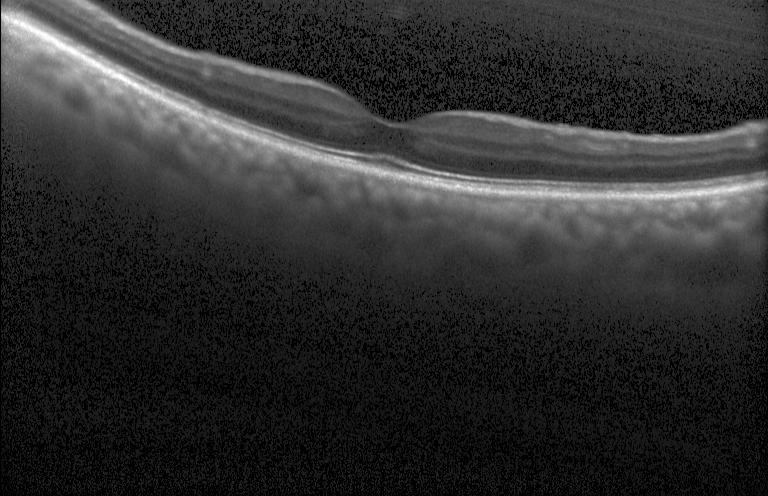 Diagnosis: no evidence of choroidal neovascularization, diabetic macular edema, or drusen.